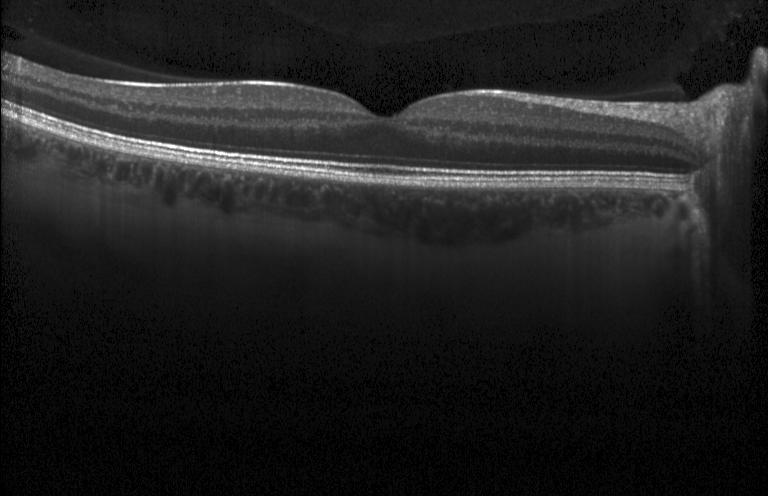 Optical coherence tomography scan · through the macula · Heidelberg Spectralis.
Dx: no choroidal neovascularization, diabetic macular edema, or drusen.